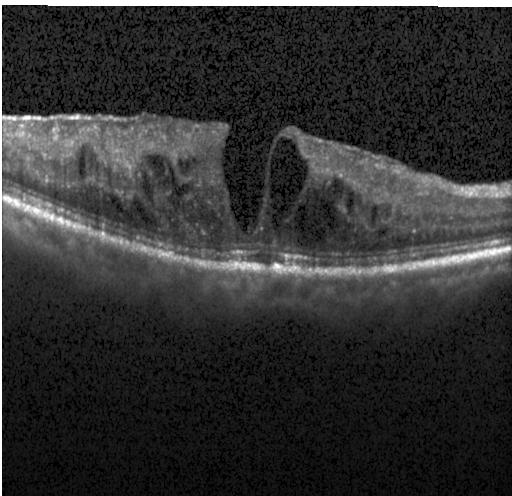

The scan shows diabetic macular edema.